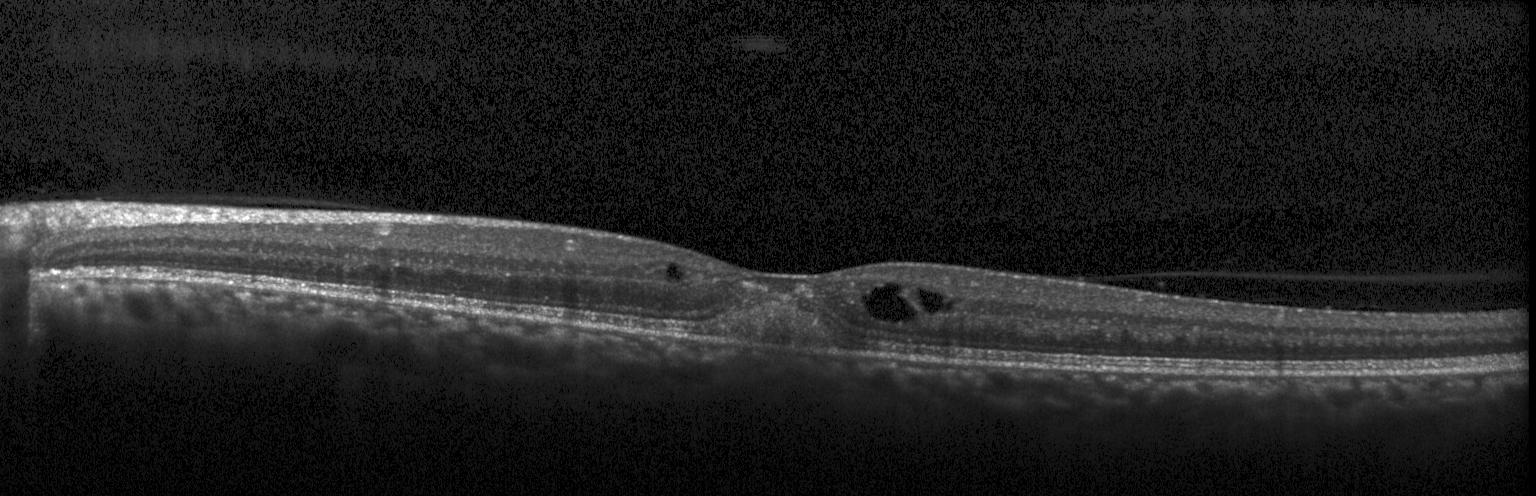 Fovea-centered · retinal OCT B-scan · acquired on a Heidelberg Spectralis · spectral-domain optical coherence tomography.
Finding: choroidal neovascularization.